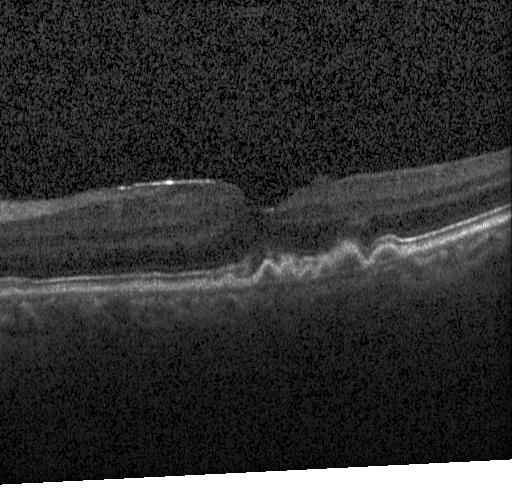
Retinal OCT B-scan · spectral-domain optical coherence tomography · macular scan · Heidelberg Spectralis OCT system.
This B-scan demonstrates drusen.